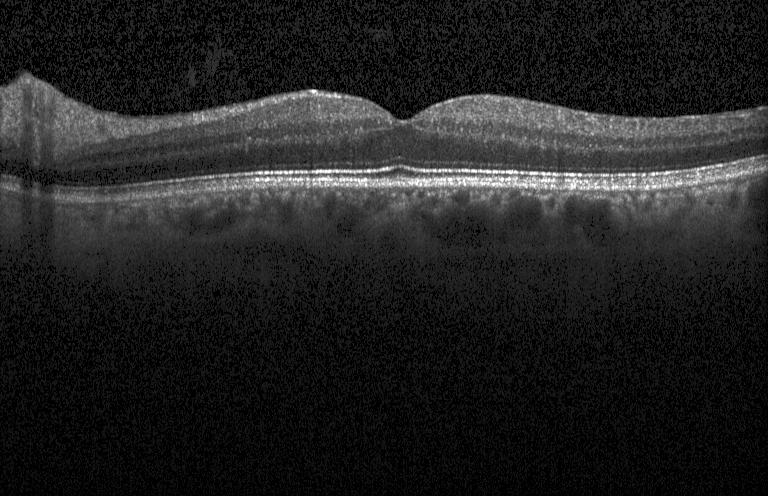 Optical coherence tomography B-scan. Spectral-domain OCT
The scan shows no choroidal neovascularization, no diabetic macular edema, and no drusen.